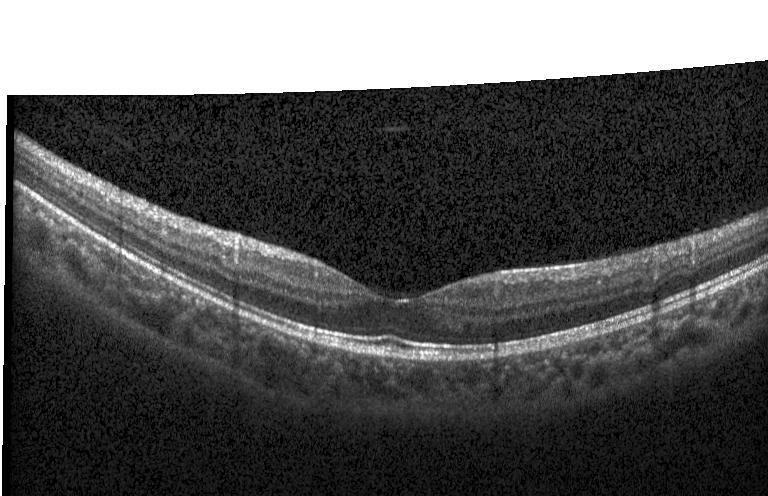

Impression: no evidence of choroidal neovascularization, diabetic macular edema, or drusen.